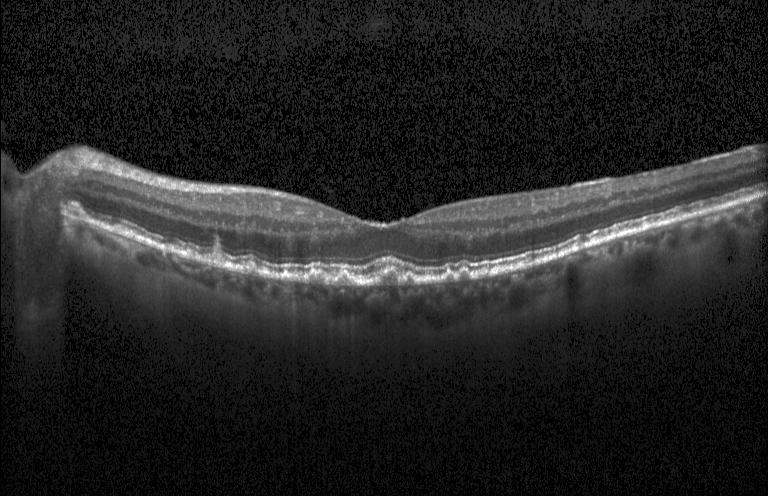

Optical coherence tomography scan; through the macula.
The scan shows sub-RPE drusenoid deposits.